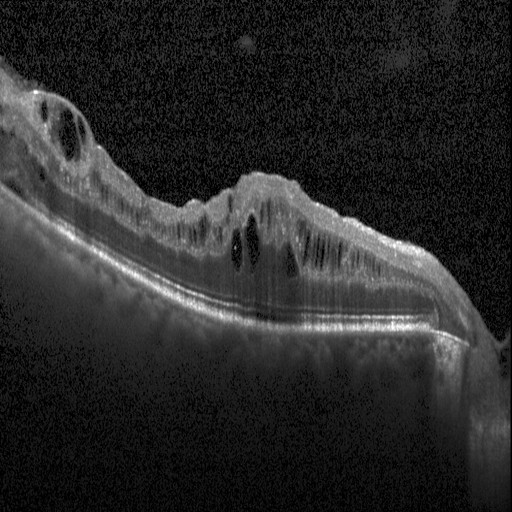 Spectral-domain OCT B-scan: DME.